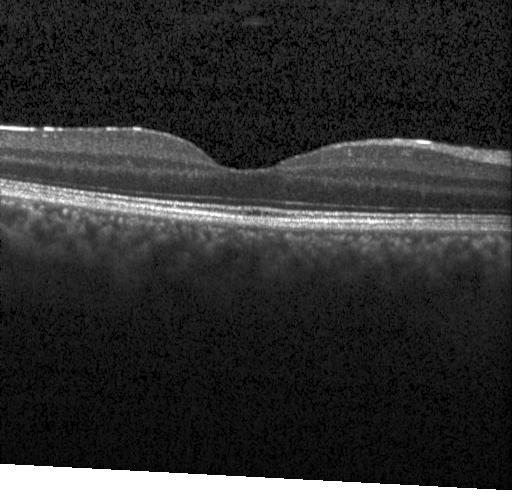 Macular OCT demonstrating no choroidal neovascularization, diabetic macular edema, or drusen.